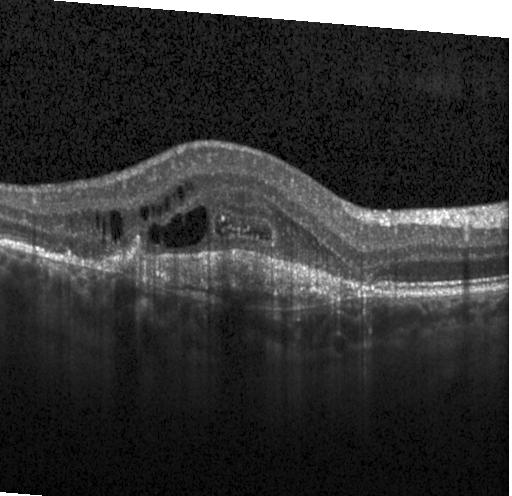 Retinal OCT B-scan — Macular OCT: a choroidal neovascular membrane.